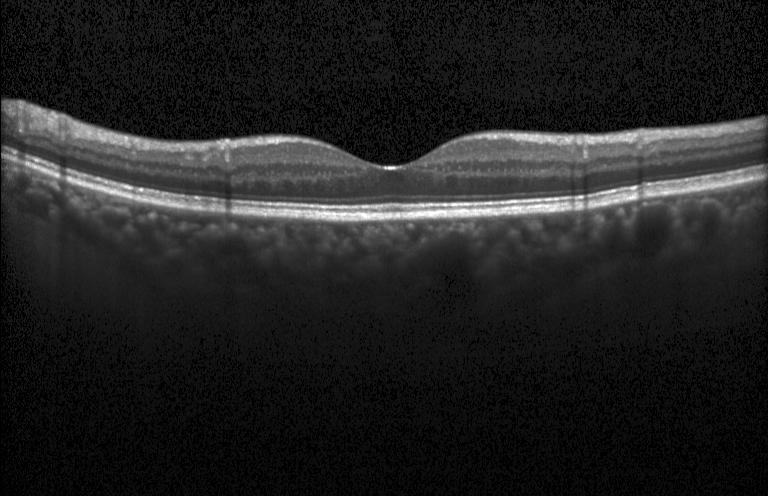

Heidelberg Spectralis OCT system · fovea-centered · retinal OCT cross-section.
Finding: neither CNV, DME, nor drusen.